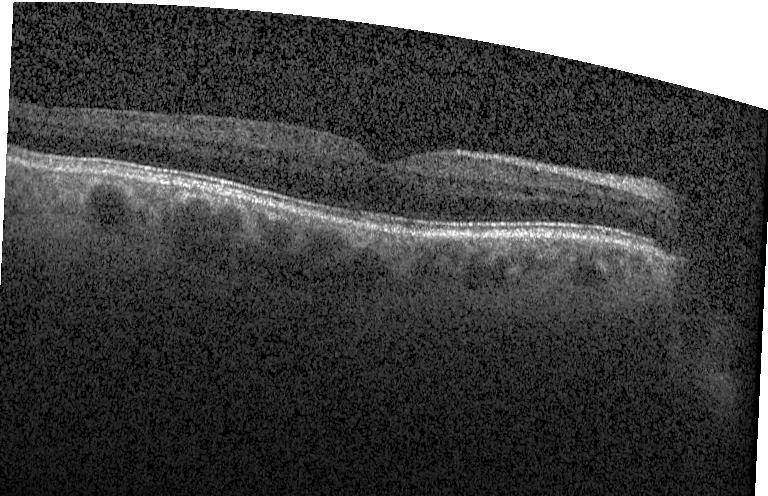
Spectral-domain OCT B-scan: no choroidal neovascularization, no diabetic macular edema, and no drusen.